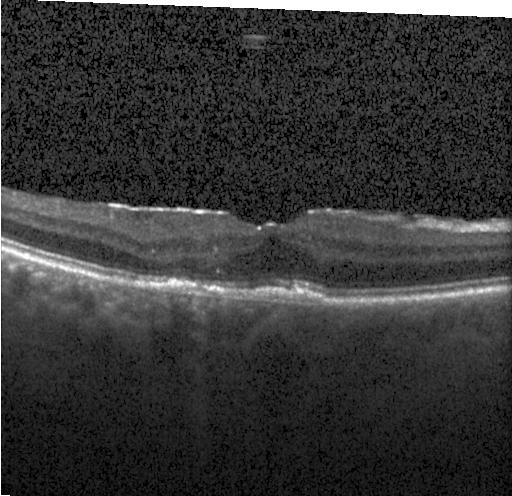
OCT scan showing CNV.